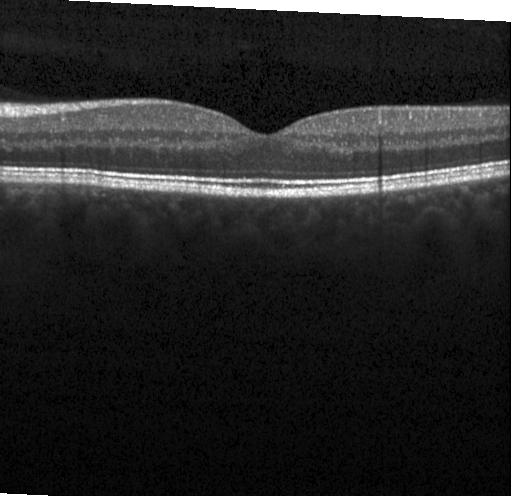

This B-scan demonstrates no choroidal neovascularization, no diabetic macular edema, and no drusen.